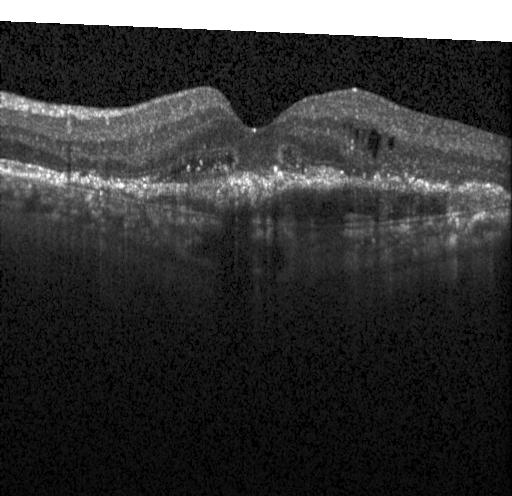
Optical coherence tomography B-scan.
Finding: choroidal neovascularization.